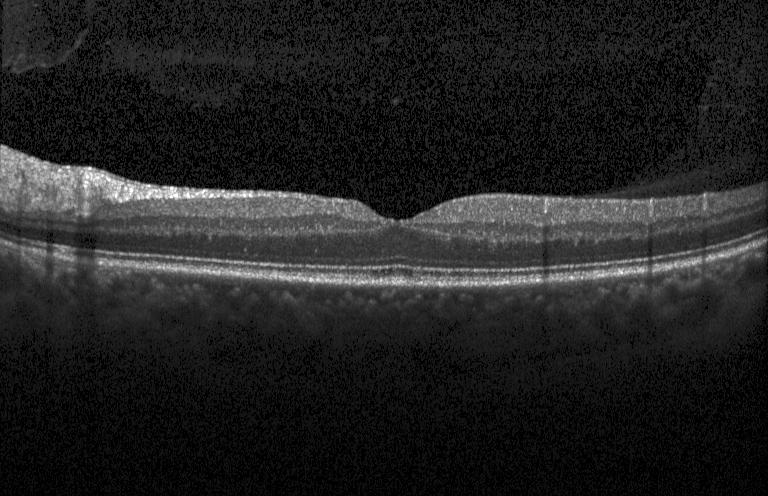 Retinal OCT cross-section; through the macula; SD-OCT
Finding: no evidence of CNV, DME, or drusen.